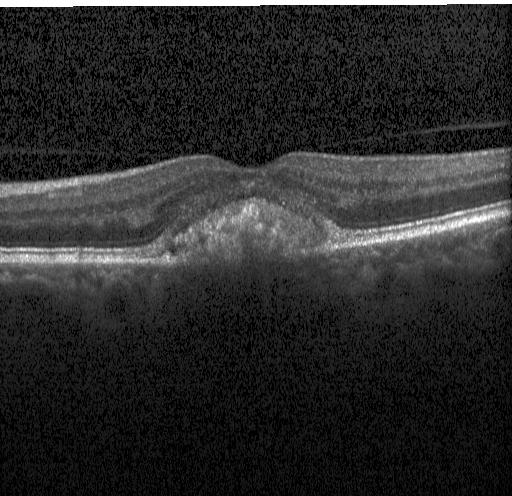 OCT finding: choroidal neovascularization (CNV).